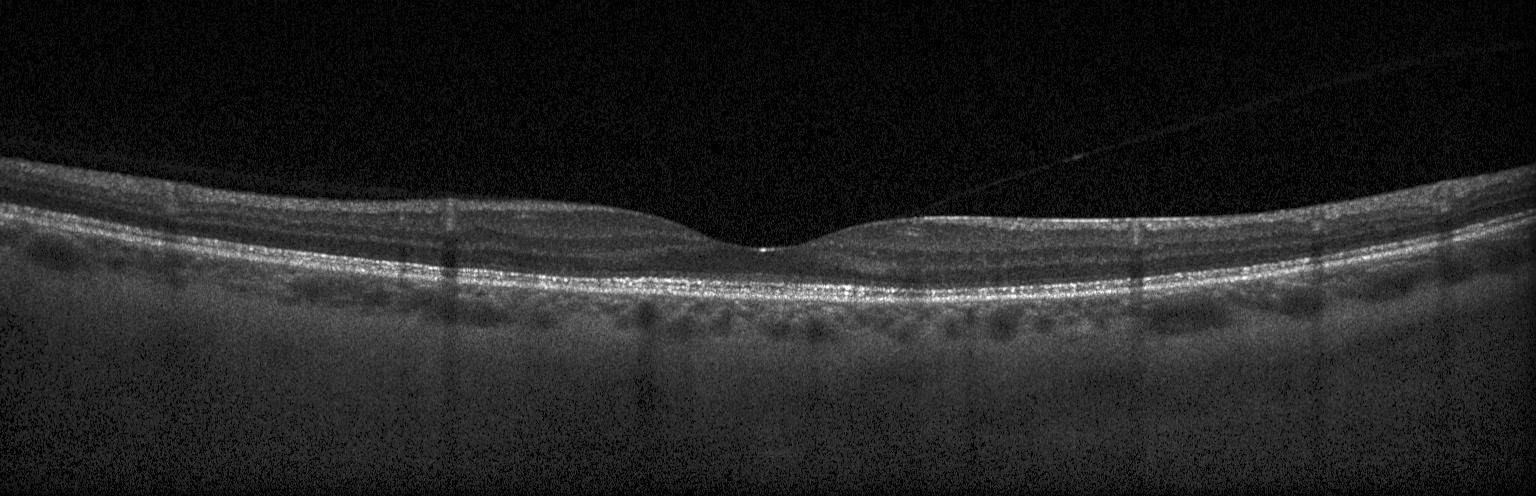 The scan shows no evidence of choroidal neovascularization, diabetic macular edema, or drusen.